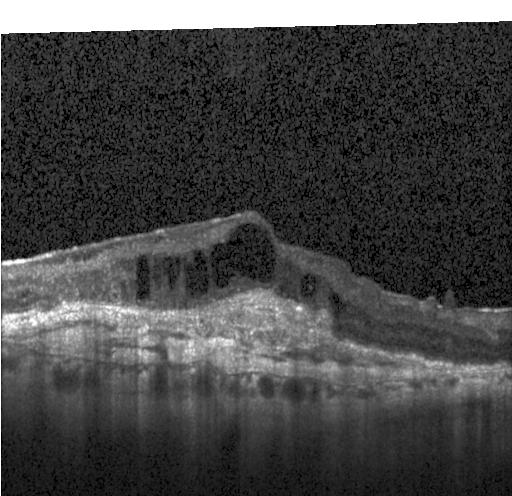 SD-OCT, optical coherence tomography B-scan, acquired on a Heidelberg Spectralis — Assessment: choroidal neovascularization (CNV).